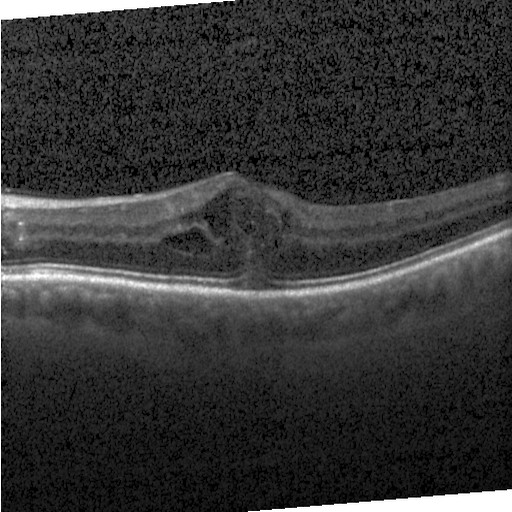

Retinal OCT cross-section showing diabetic macular edema (DME).